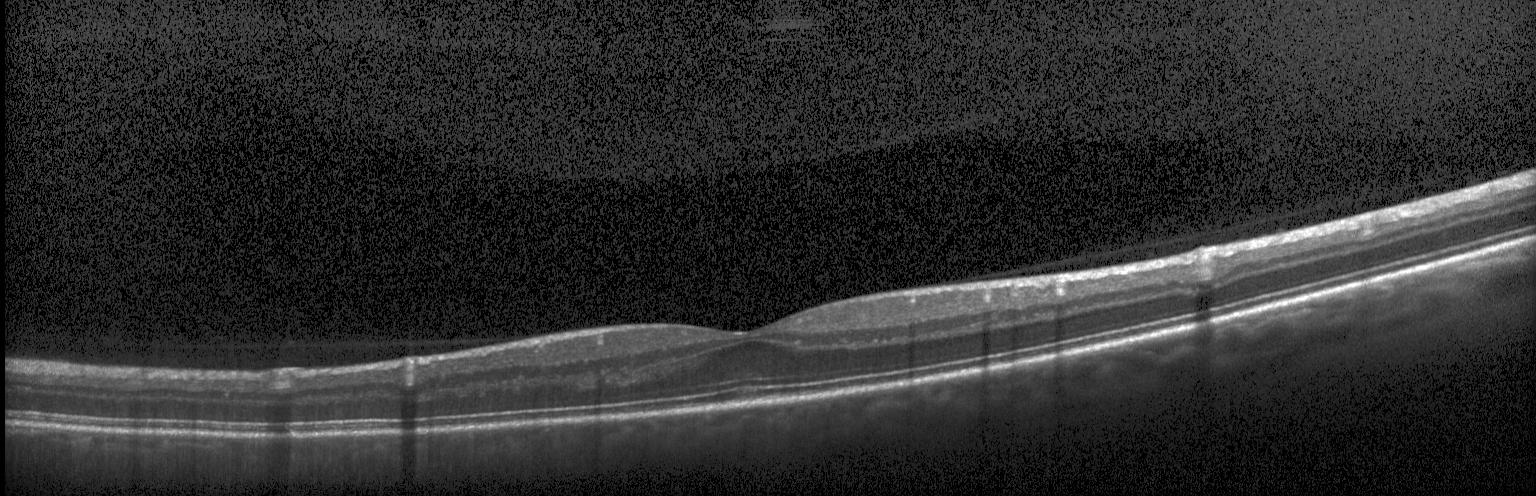
Spectral-domain optical coherence tomography. Optical coherence tomography B-scan.
Impression: no choroidal neovascularization, diabetic macular edema, or drusen.